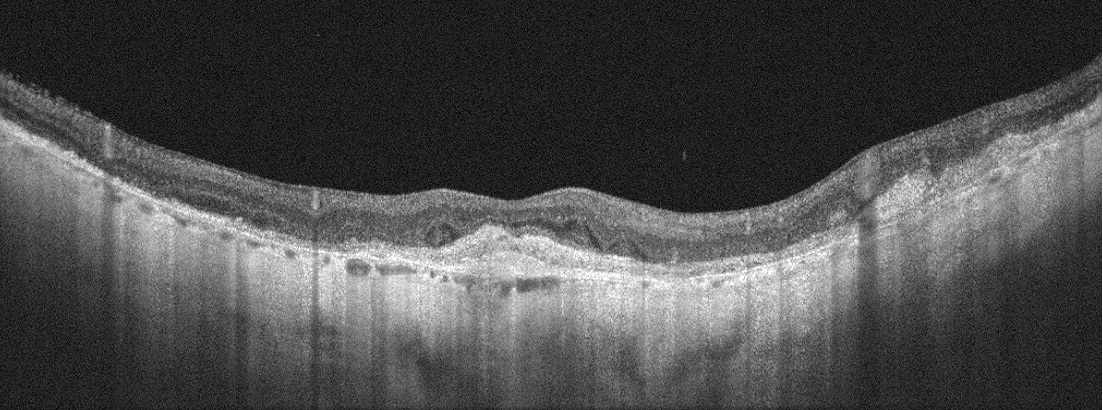 OCT finding: age-related macular degeneration.